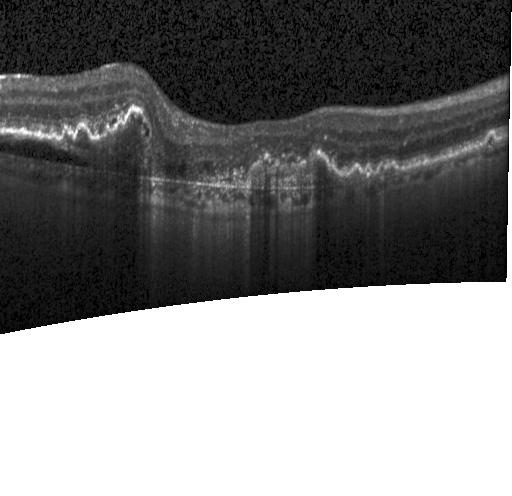

OCT B-scan, Heidelberg Spectralis — Finding: choroidal neovascularization.